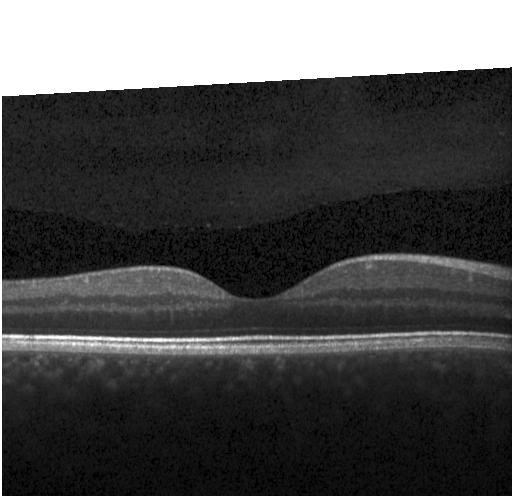 Finding: no choroidal neovascularization, diabetic macular edema, or drusen.